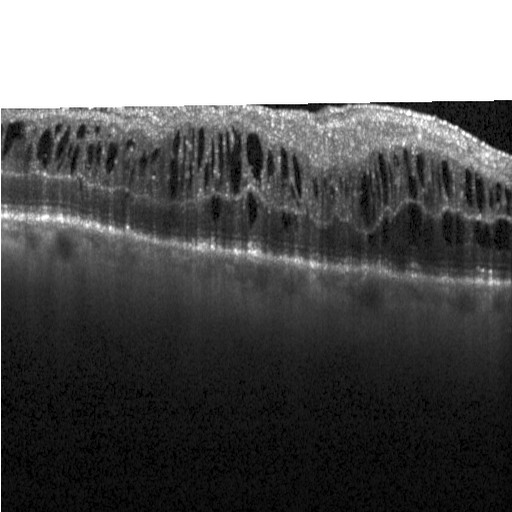

OCT B-scan, centered on the fovea, acquired on a Heidelberg Spectralis.
Finding: DME.